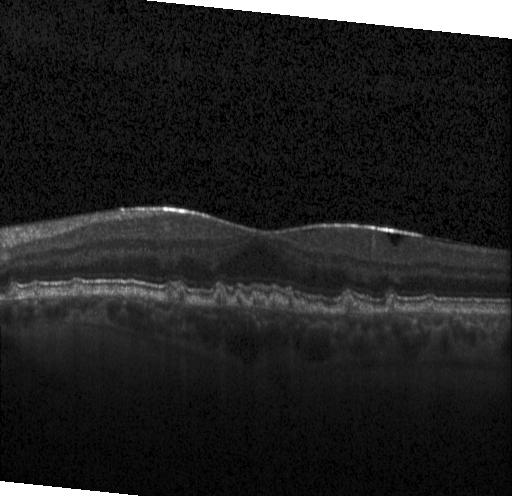 OCT B-scan showing multiple drusen.